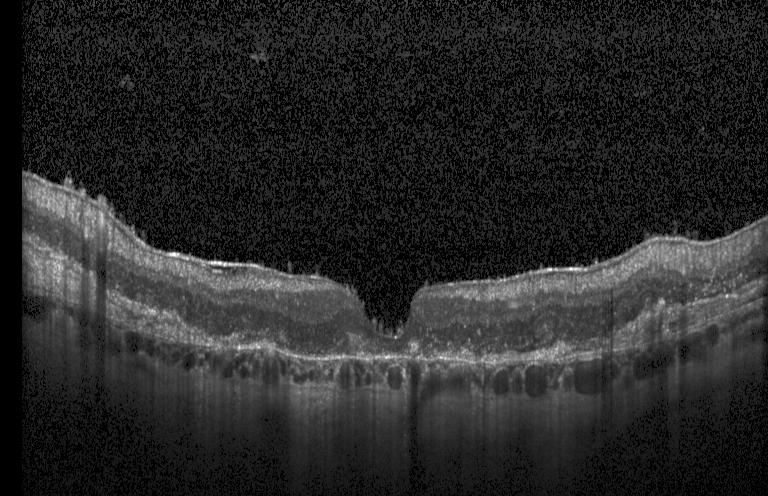
Retinal OCT B-scan. Assessment: a choroidal neovascular membrane.